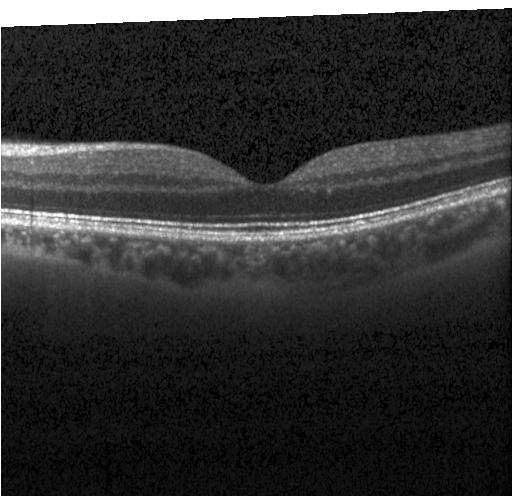 Macular OCT demonstrating no evidence of choroidal neovascularization, diabetic macular edema, or drusen.